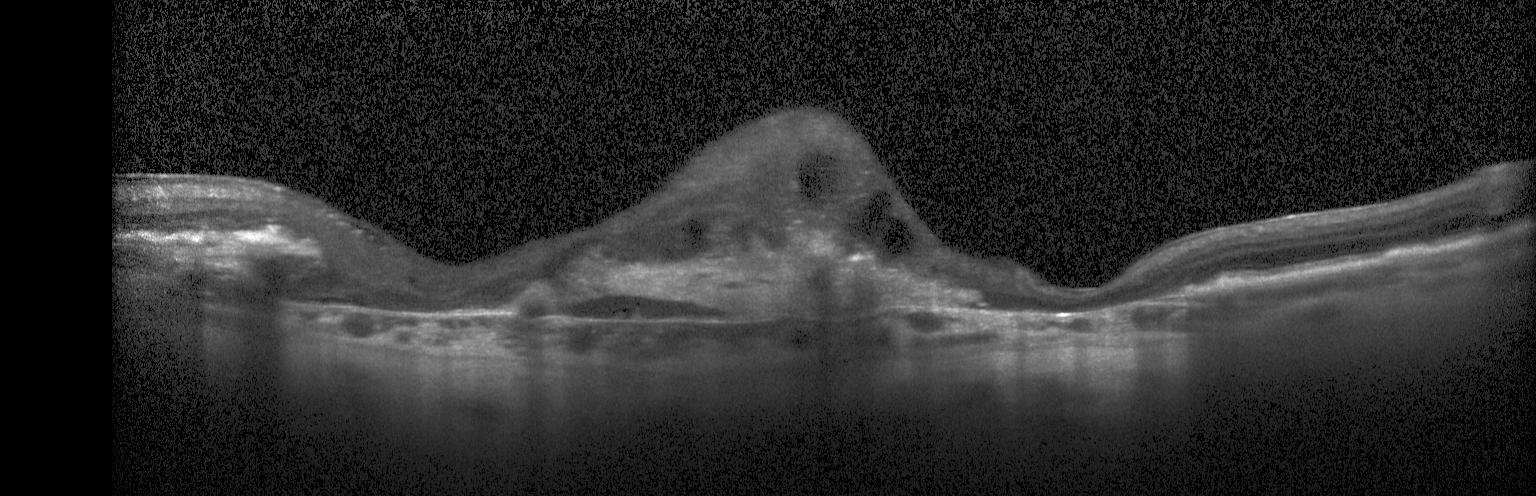

Optical coherence tomography B-scan.
Diagnosis: choroidal neovascularization.